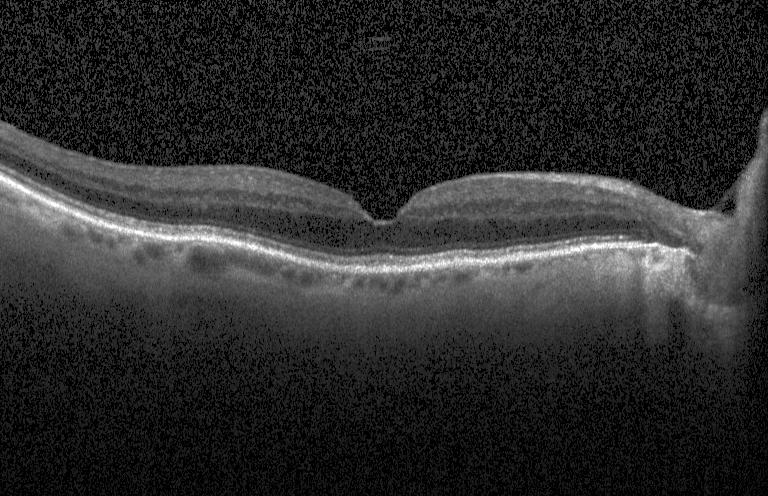 Diagnosis: no evidence of choroidal neovascularization, diabetic macular edema, or drusen.